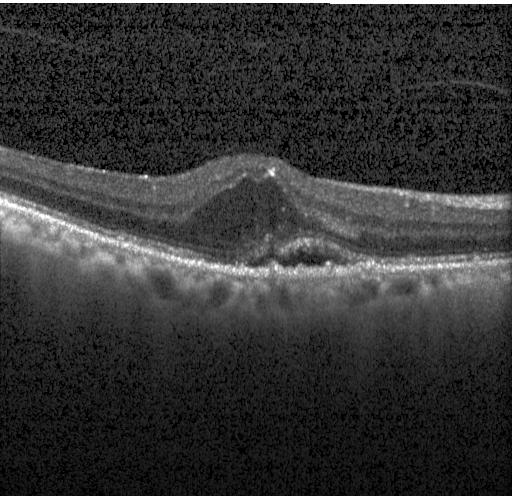

Retinal OCT cross-section · centered on the fovea · spectral-domain optical coherence tomography — Diagnosis: a choroidal neovascular membrane.